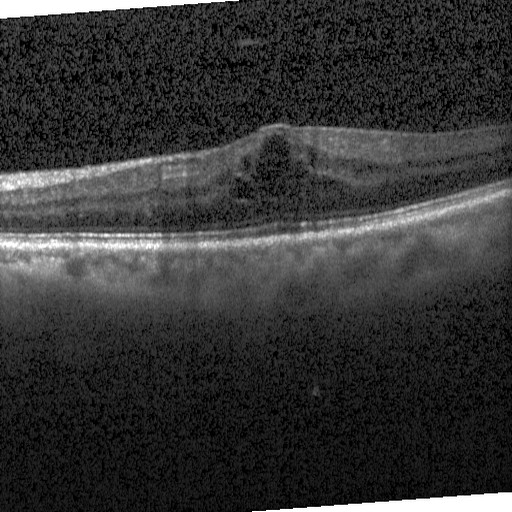 Finding: DME.